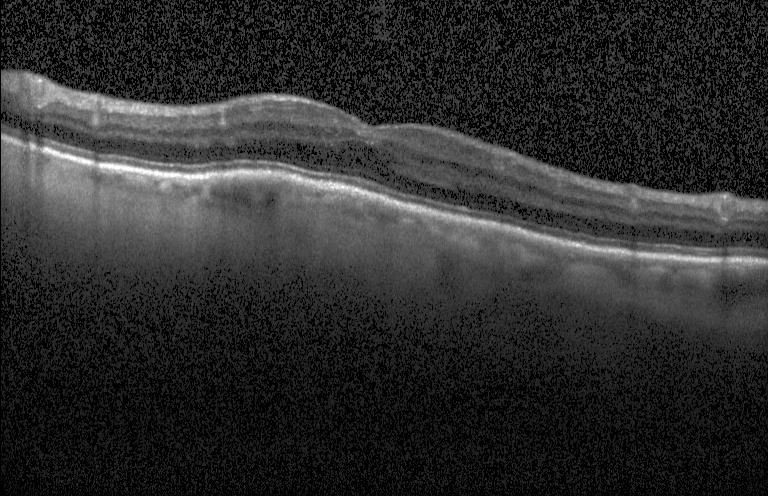

Retinal OCT cross-section.
Macular OCT: no choroidal neovascularization, diabetic macular edema, or drusen.